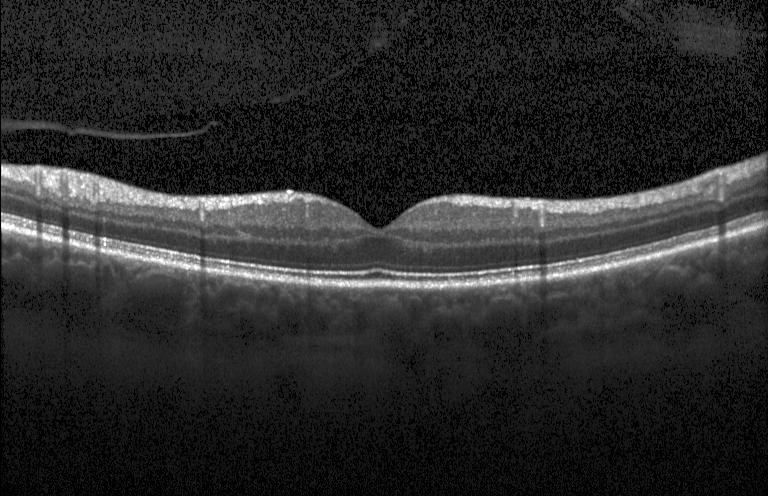

Optical coherence tomography scan; spectral-domain optical coherence tomography.
OCT finding: no CNV, no DME, and no drusen.